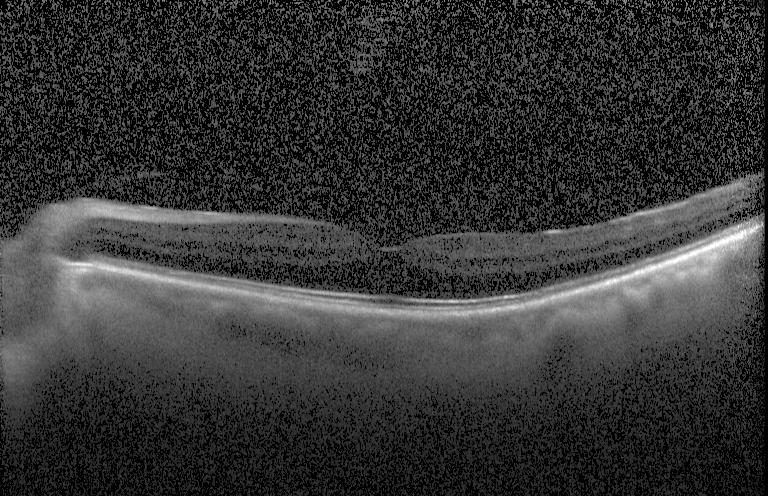 Spectral-domain OCT. Macular scan. Retinal OCT B-scan — Finding: no choroidal neovascularization, diabetic macular edema, or drusen.